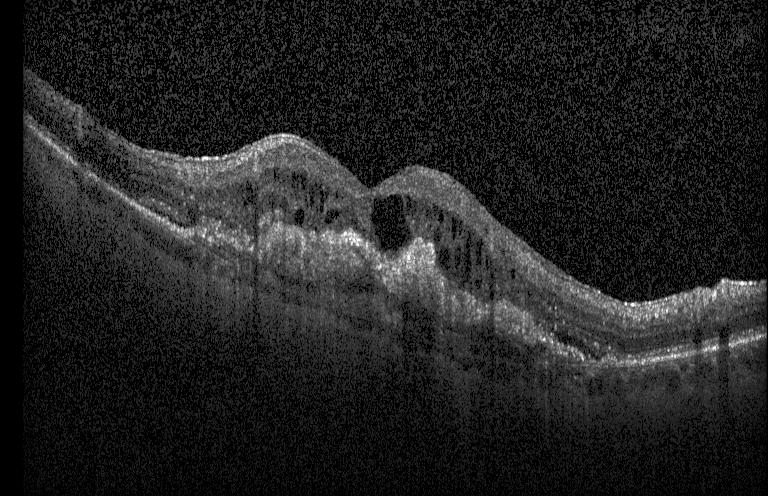 Fovea-centered, SD-OCT, retinal OCT B-scan — This B-scan demonstrates CNV.